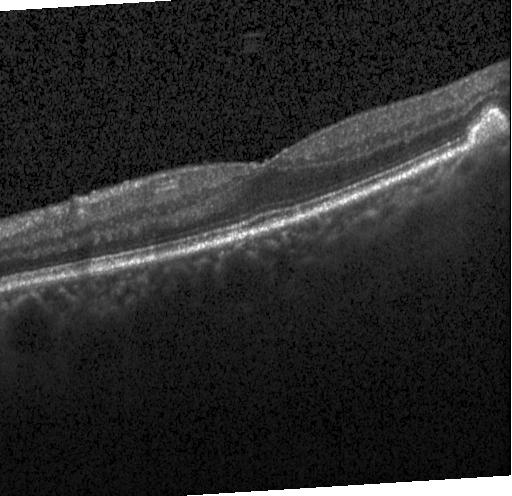
Optical coherence tomography B-scan. Finding: sub-RPE drusenoid deposits.